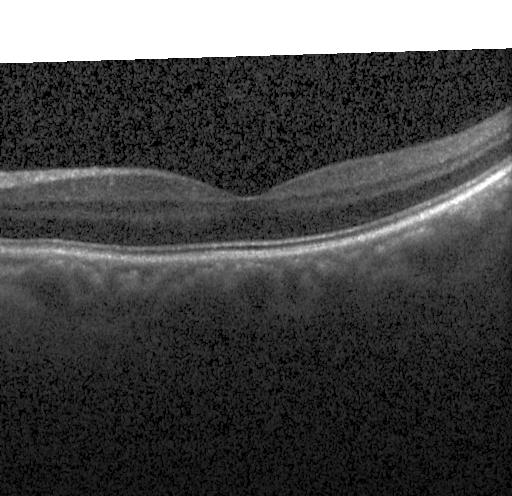
Heidelberg Spectralis OCT system; OCT B-scan — Finding: neither CNV, DME, nor drusen.